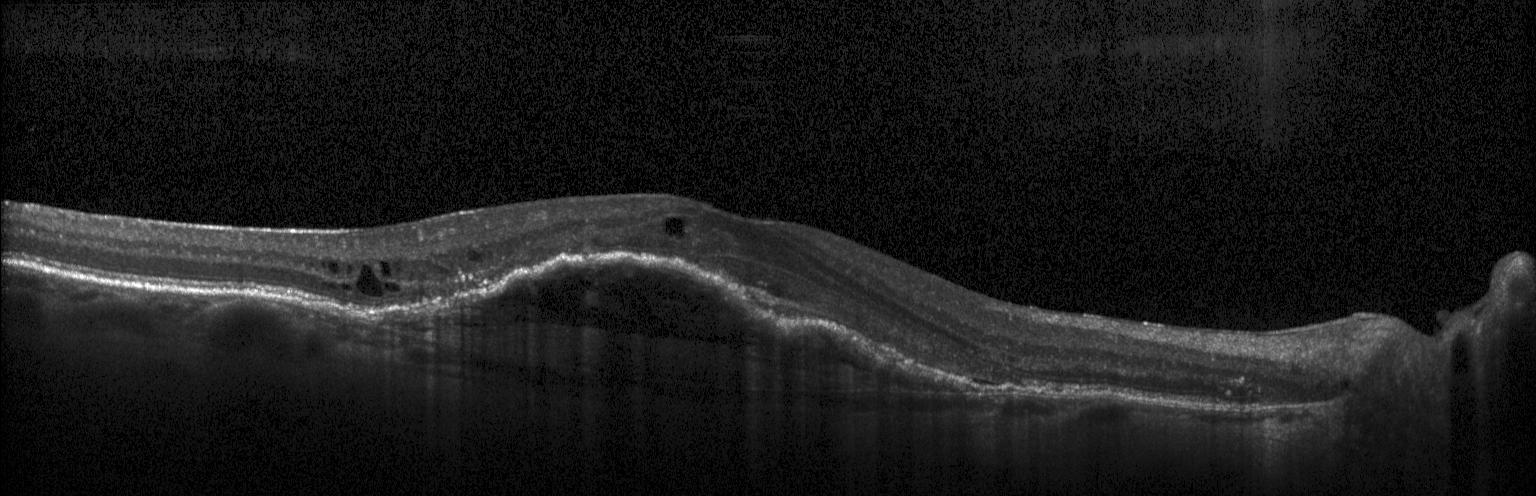

Optical coherence tomography scan — The scan shows a choroidal neovascular membrane.